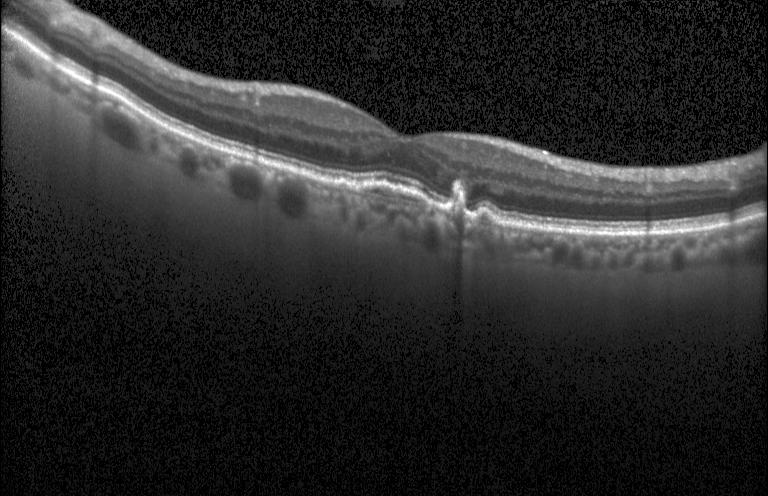

Assessment: choroidal neovascularization (CNV).